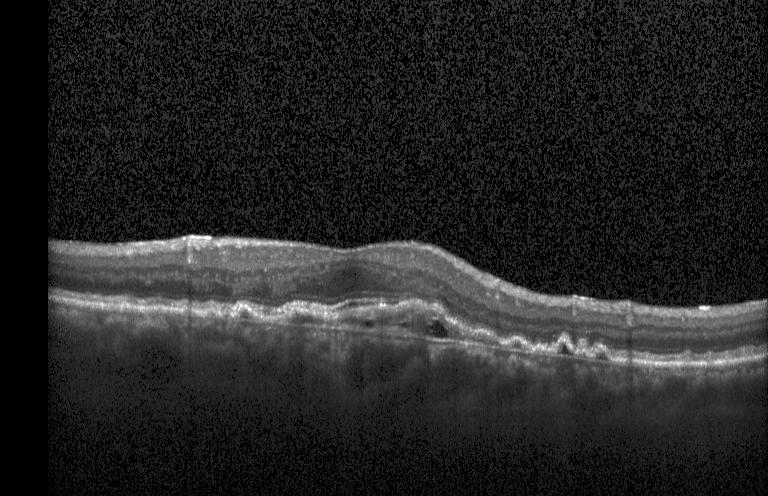

Spectral-domain optical coherence tomography; optical coherence tomography scan; macular scan. A choroidal neovascular membrane.